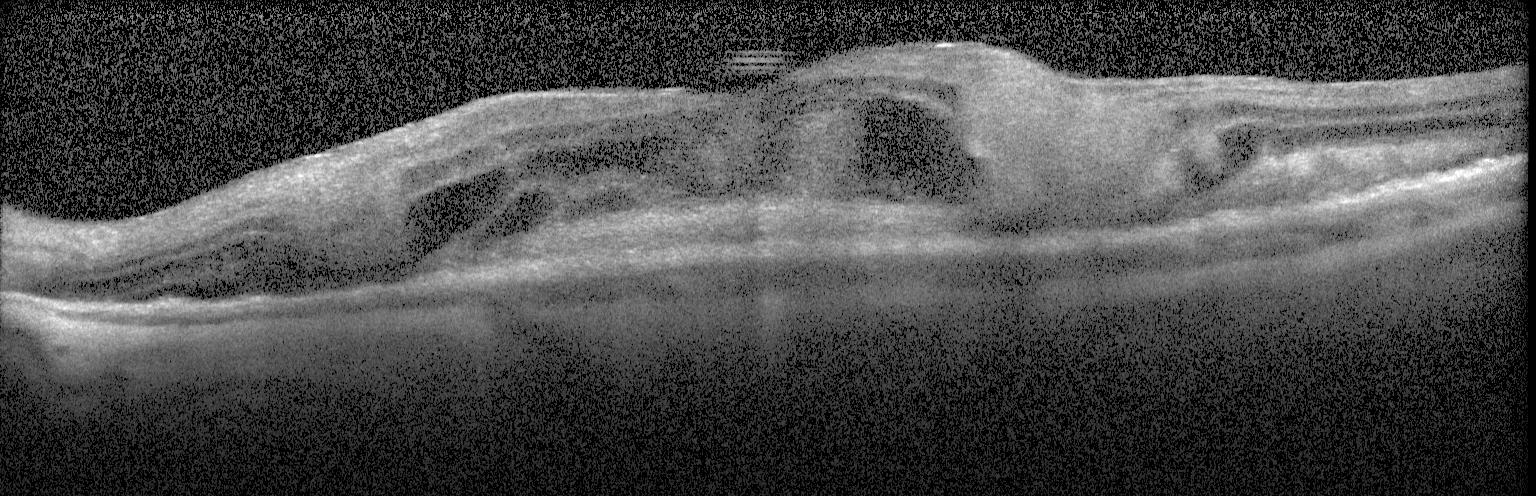
Retinal OCT cross-section; Heidelberg Spectralis
This B-scan demonstrates choroidal neovascularization (CNV).